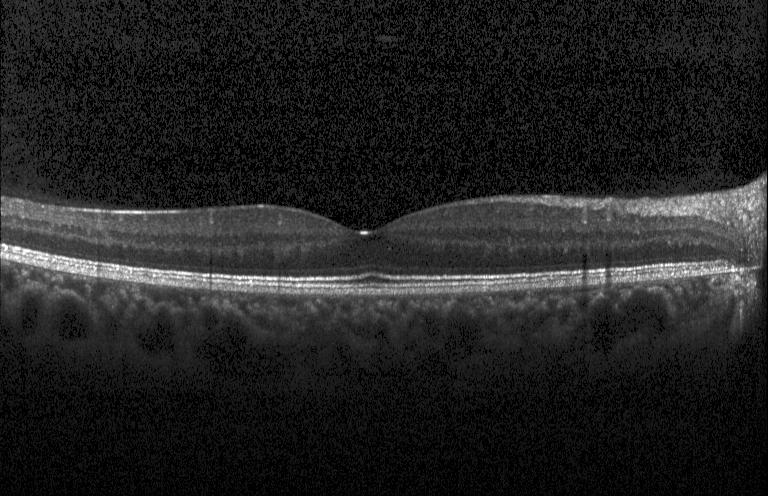

OCT finding: no choroidal neovascularization, no diabetic macular edema, and no drusen.